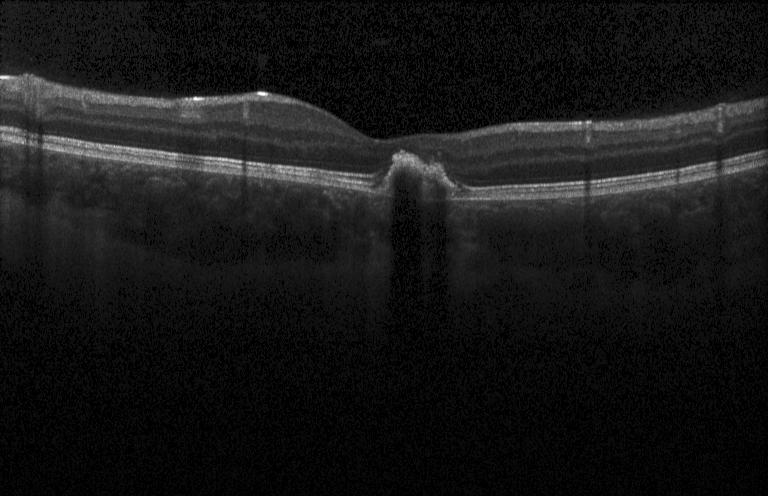

Optical coherence tomography B-scan
Finding: a choroidal neovascular membrane.